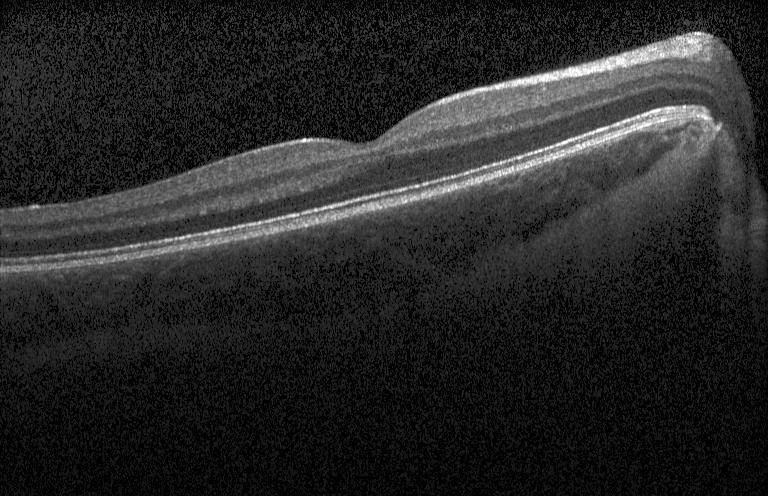
Optical coherence tomography B-scan — No choroidal neovascularization, diabetic macular edema, or drusen.